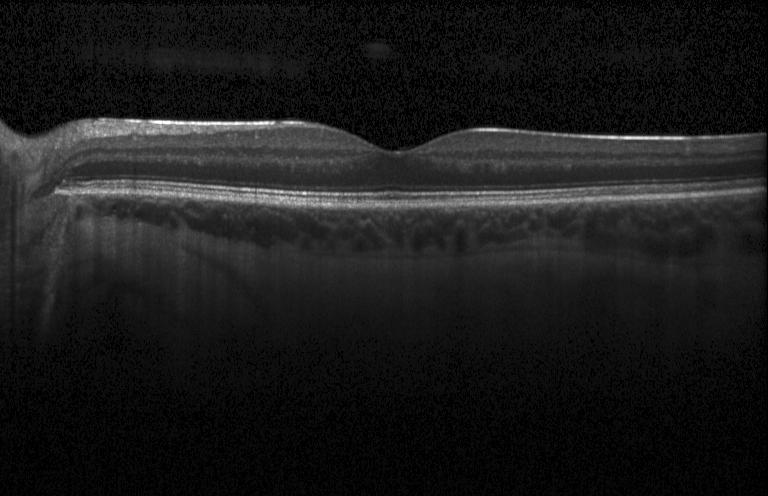
Heidelberg Spectralis OCT system · optical coherence tomography scan.
Dx: no CNV, DME, or drusen.